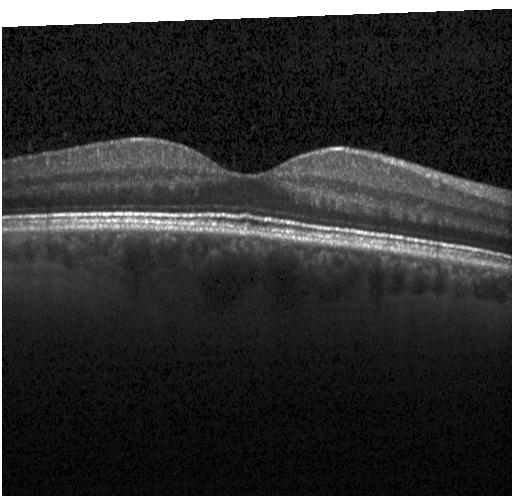 Retinal OCT B-scan — Dx: neither CNV, DME, nor drusen.